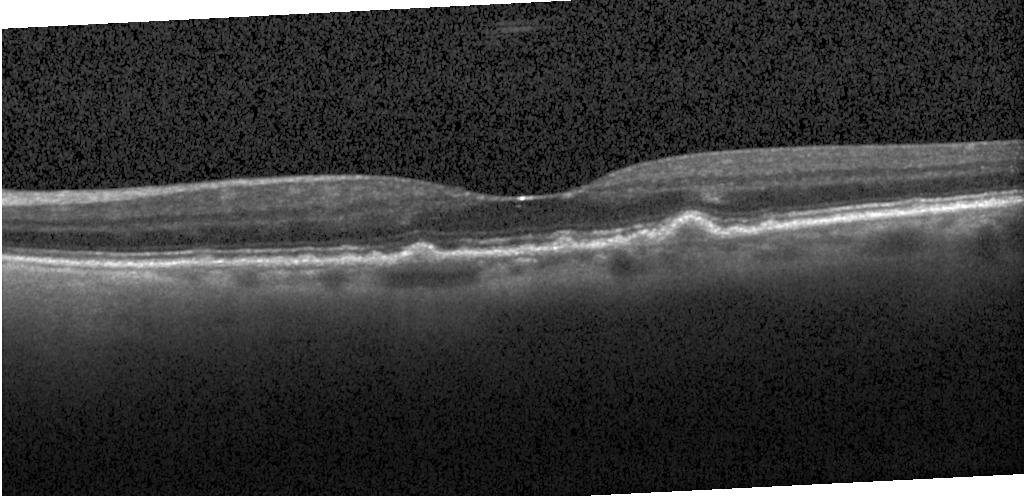 Instrument: Heidelberg Spectralis · OCT line scan.
Impression: multiple drusen.